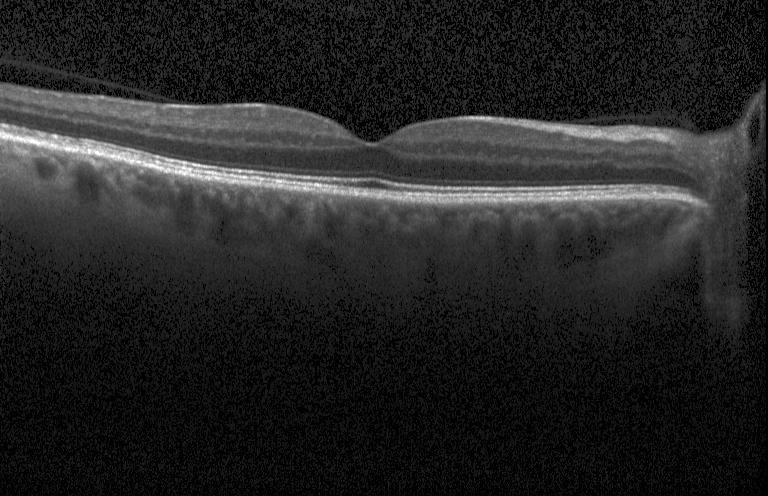 Heidelberg Spectralis, optical coherence tomography B-scan, spectral-domain optical coherence tomography, centered on the fovea
Dx: no choroidal neovascularization, no diabetic macular edema, and no drusen.